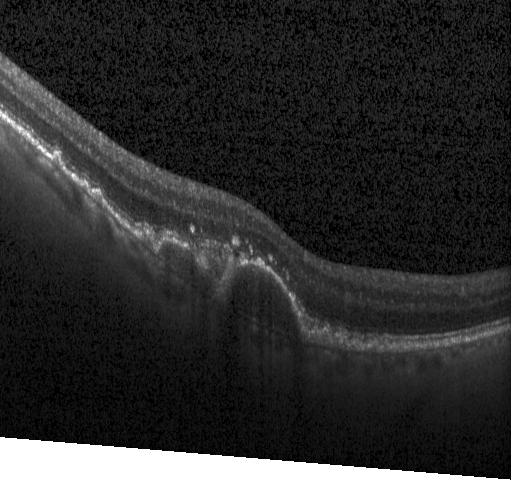
Retinal OCT cross-section
A choroidal neovascular membrane.